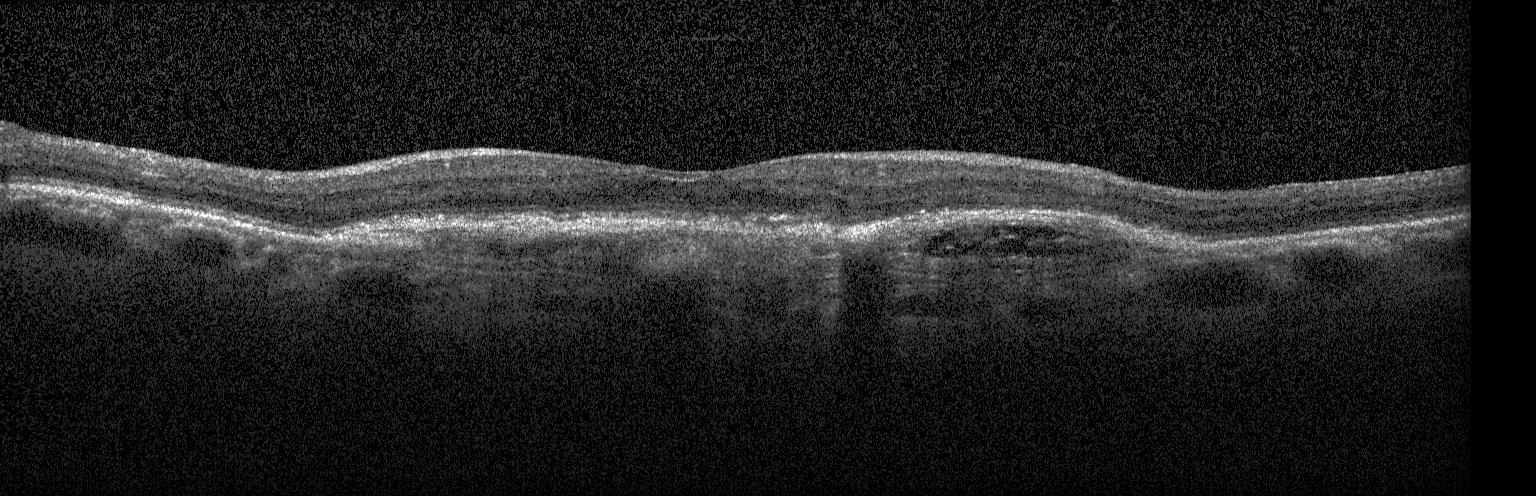
Finding: choroidal neovascularization (CNV).